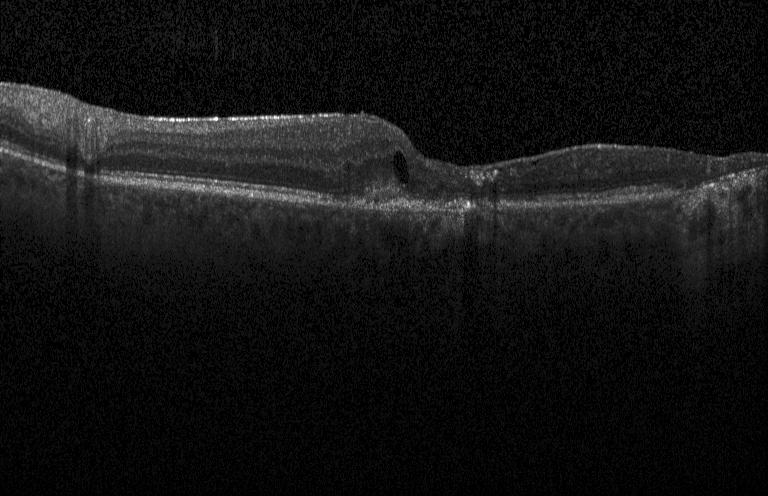 This B-scan demonstrates choroidal neovascularization (CNV).